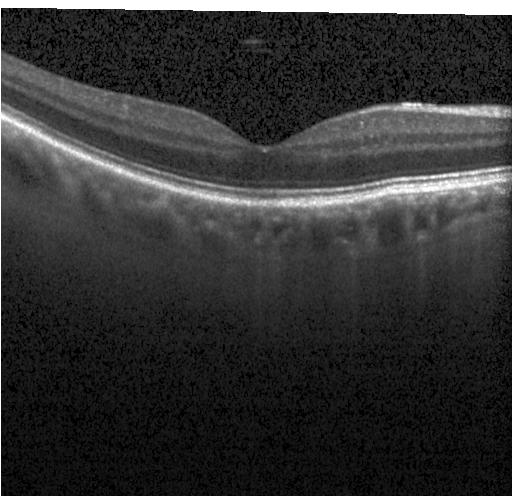 Heidelberg Spectralis OCT system · SD-OCT · optical coherence tomography B-scan · horizontal scan through the fovea — Assessment: no choroidal neovascularization, no diabetic macular edema, and no drusen.